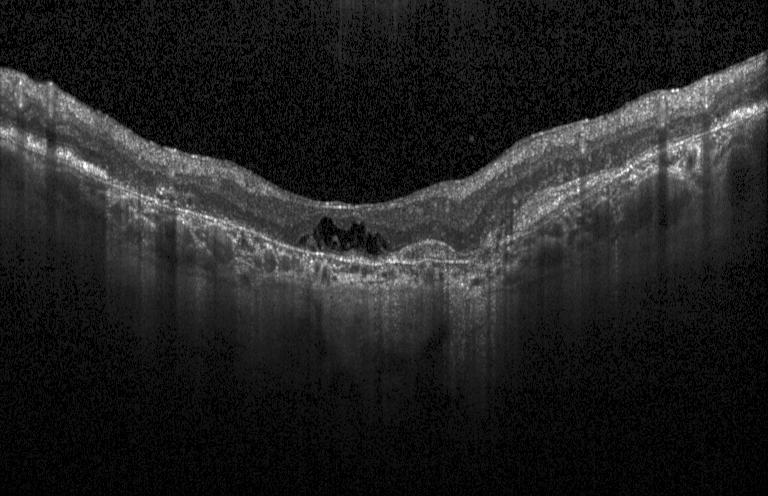

Heidelberg Spectralis OCT system; OCT B-scan; horizontal scan through the fovea.
Diagnosis: a choroidal neovascular membrane.